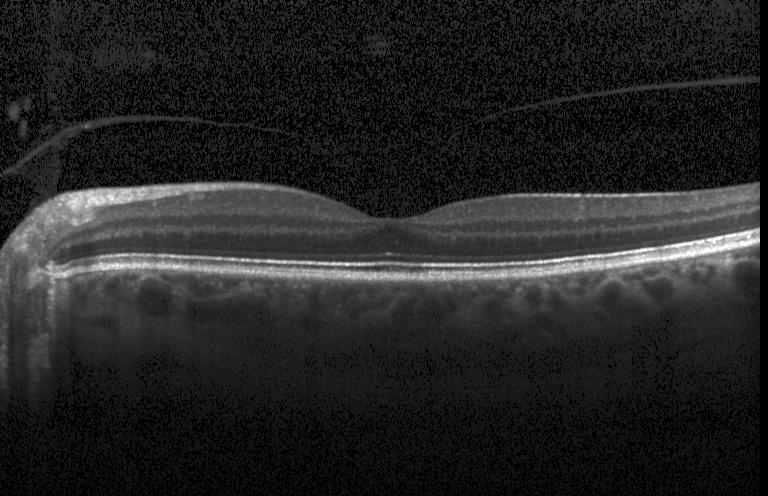

Optical coherence tomography B-scan
Diagnosis: no evidence of choroidal neovascularization, diabetic macular edema, or drusen.